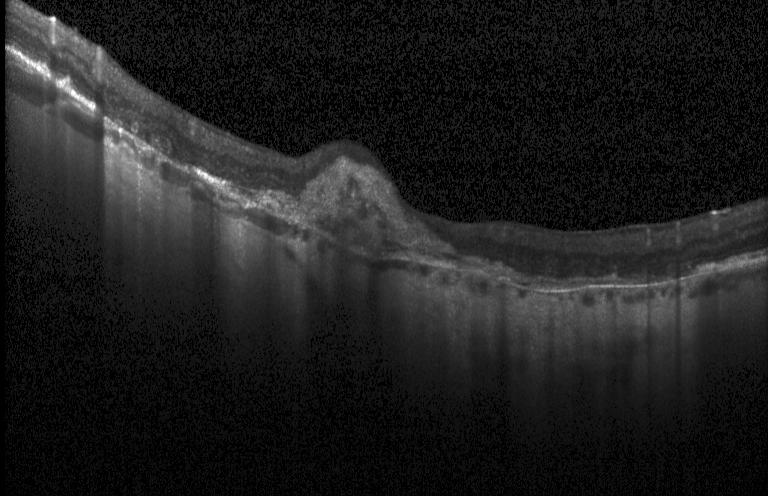
Optical coherence tomography scan. Spectral-domain OCT.
Finding: choroidal neovascularization (CNV).